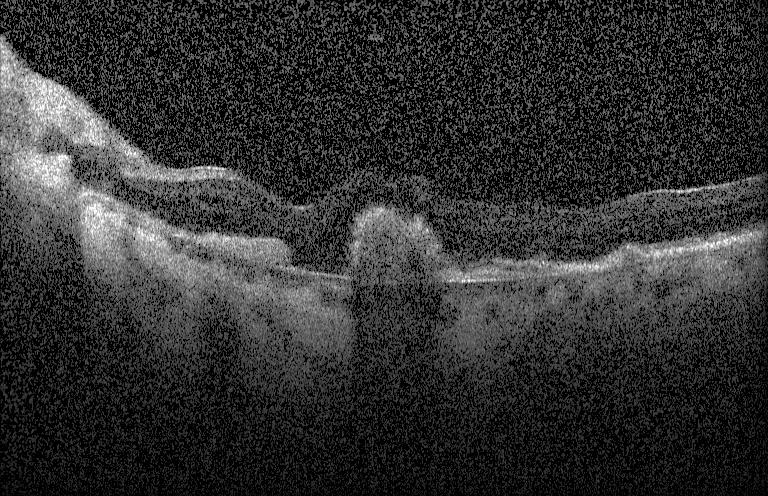

OCT B-scan, fovea-centered
Assessment: a choroidal neovascular membrane.